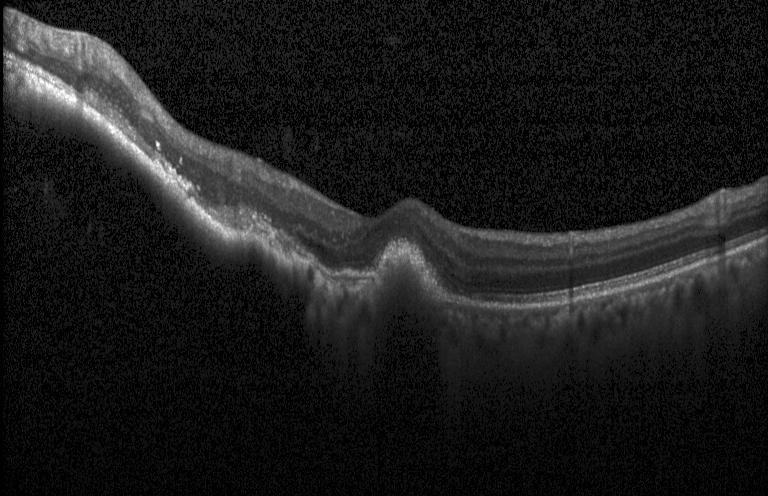

Dx: a choroidal neovascular membrane.